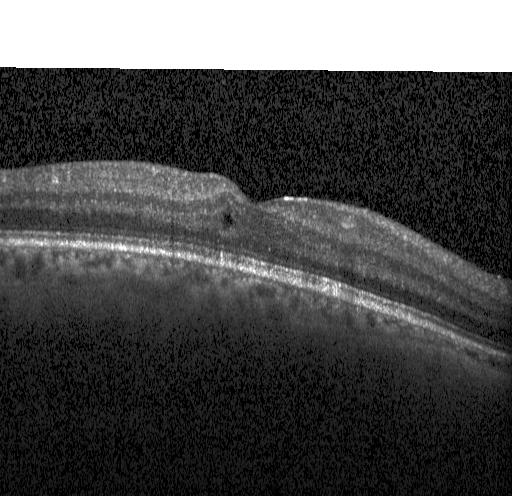 Retinal OCT cross-section, spectral-domain optical coherence tomography.
Diagnosis: DME.